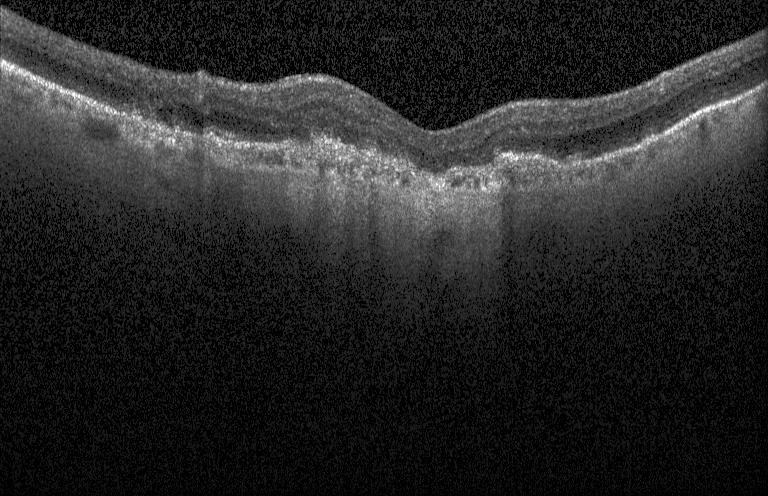

Optical coherence tomography B-scan.
Macular OCT: a choroidal neovascular membrane.